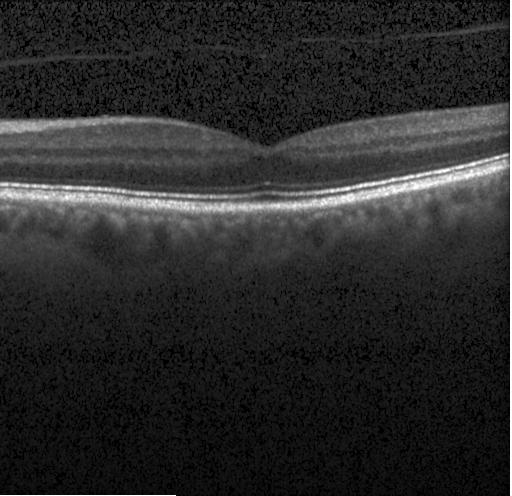 OCT finding: no evidence of choroidal neovascularization, diabetic macular edema, or drusen.